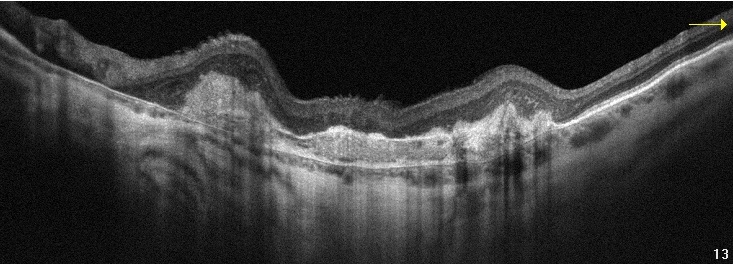
Macular OCT demonstrating age-related macular degeneration.